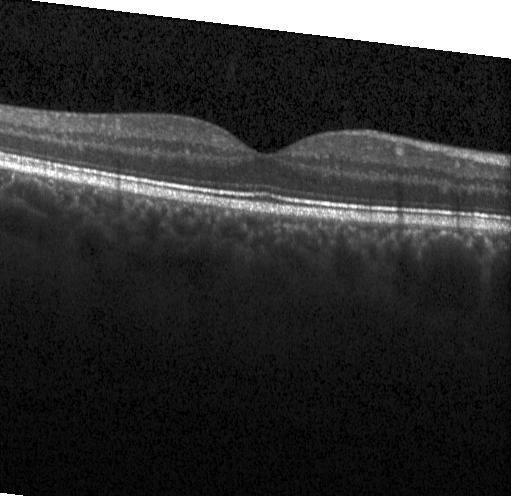 Dx: neither choroidal neovascularization, diabetic macular edema, nor drusen.